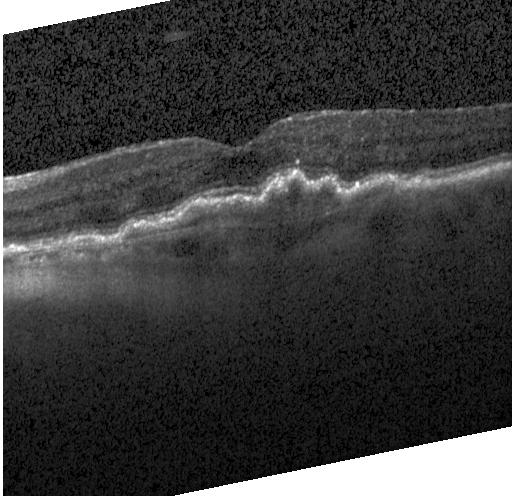 Optical coherence tomography scan.
Impression: choroidal neovascularization.